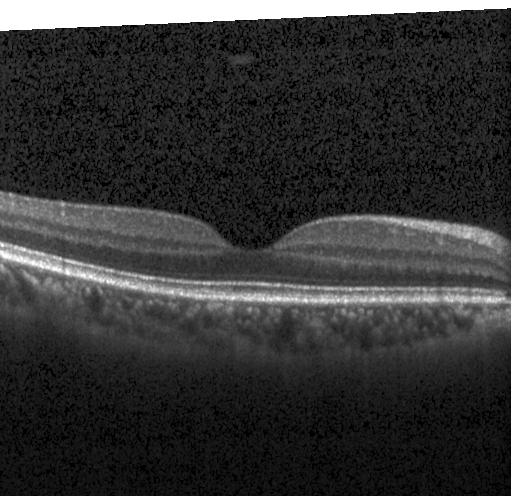
Finding: no choroidal neovascularization, diabetic macular edema, or drusen.